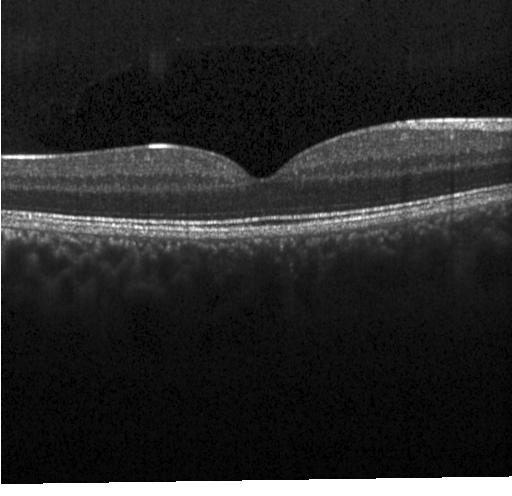 Dx: no choroidal neovascularization, no diabetic macular edema, and no drusen.